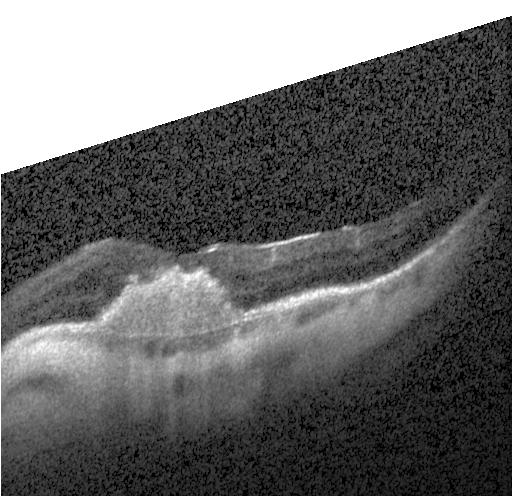

Impression: choroidal neovascularization (CNV).